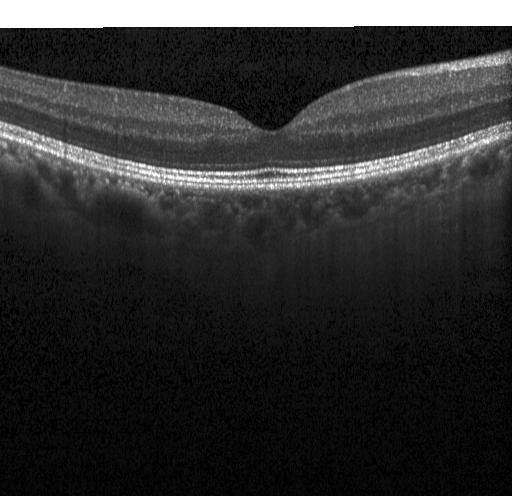 Fovea-centered · optical coherence tomography B-scan · SD-OCT · Heidelberg Spectralis. Dx: no choroidal neovascularization, no diabetic macular edema, and no drusen.